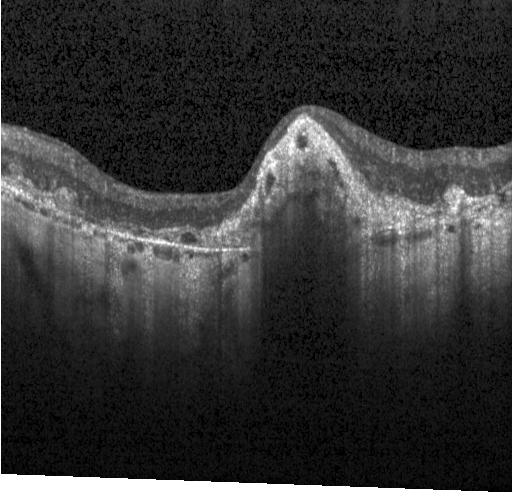

The scan shows a choroidal neovascular membrane.